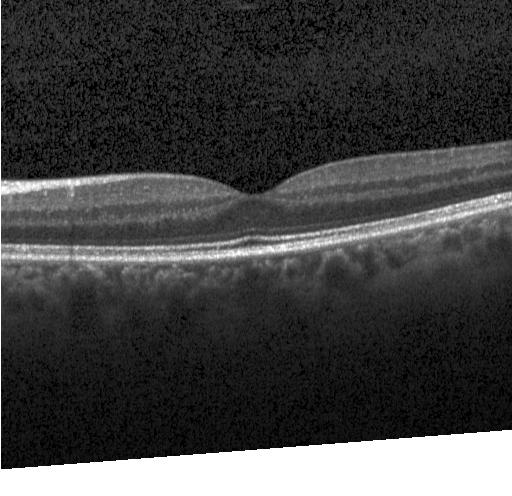

Retinal OCT cross-section.
Diagnosis: neither choroidal neovascularization, diabetic macular edema, nor drusen.